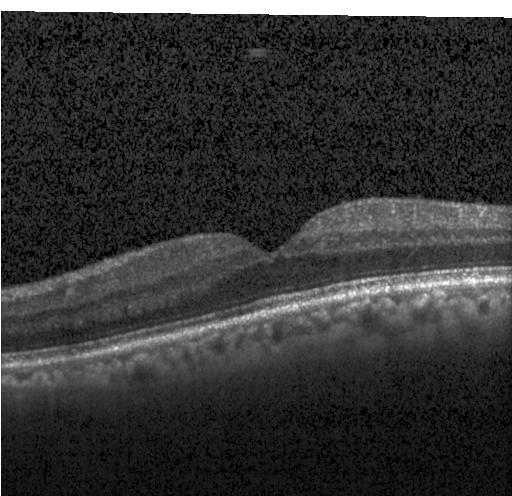

Spectral-domain OCT · retinal OCT cross-section · centered on the fovea · acquired on a Heidelberg Spectralis — No choroidal neovascularization, no diabetic macular edema, and no drusen.